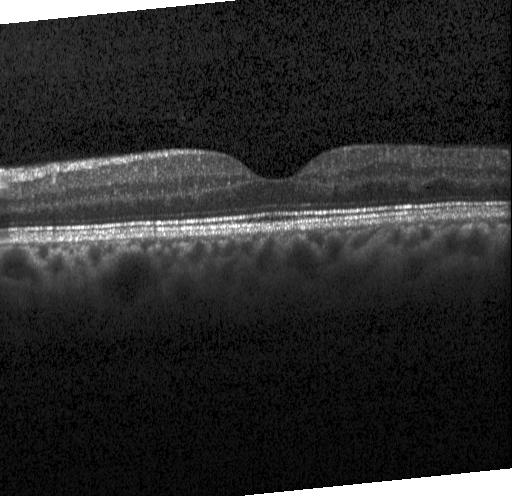

OCT finding: no choroidal neovascularization, no diabetic macular edema, and no drusen.